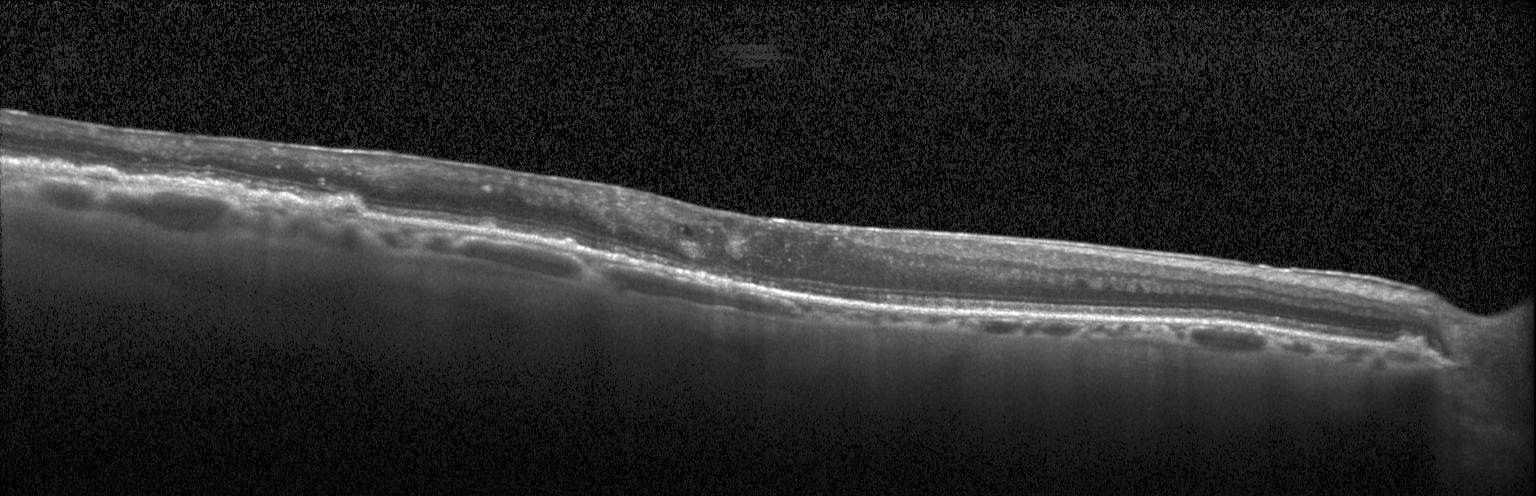 Retinal OCT cross-section showing a choroidal neovascular membrane.